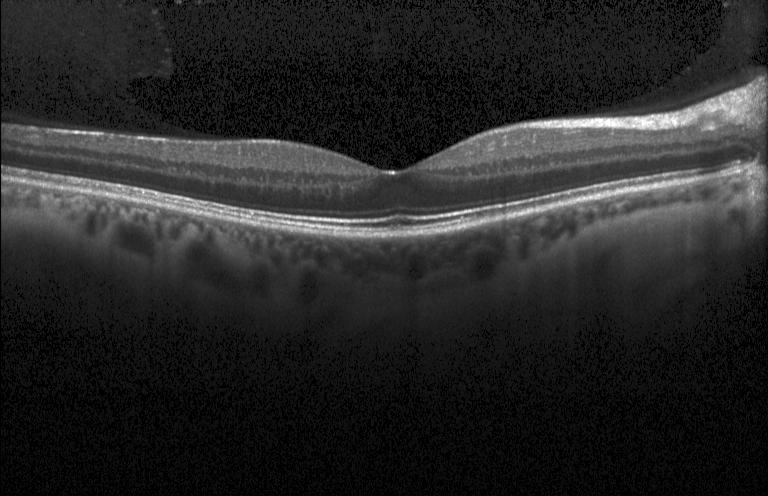 SD-OCT; OCT line scan — Assessment: no choroidal neovascularization, diabetic macular edema, or drusen.